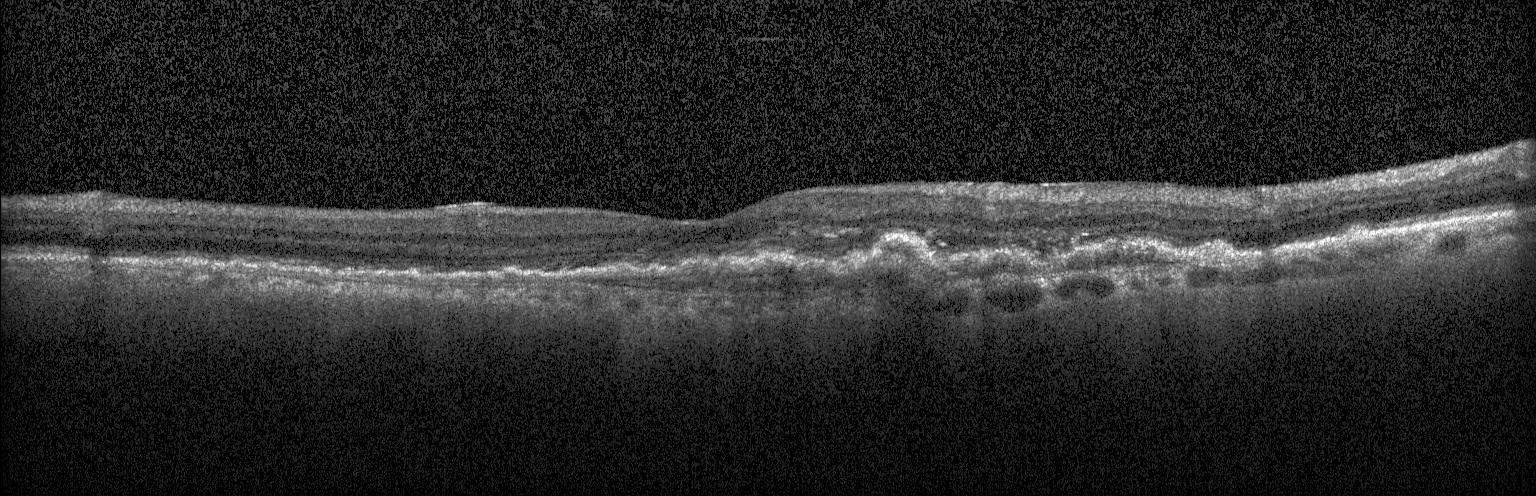 Diagnosis: choroidal neovascularization (CNV).